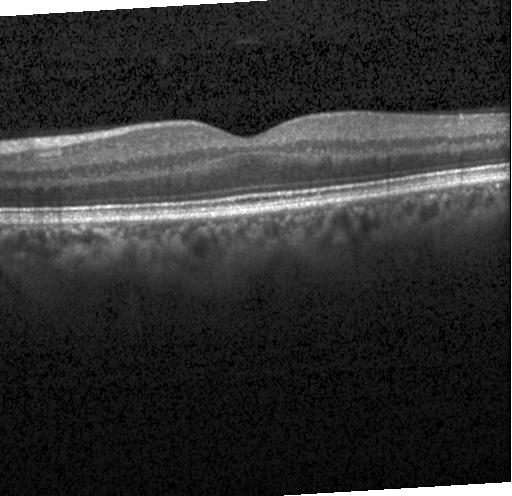 Impression: no choroidal neovascularization, no diabetic macular edema, and no drusen.